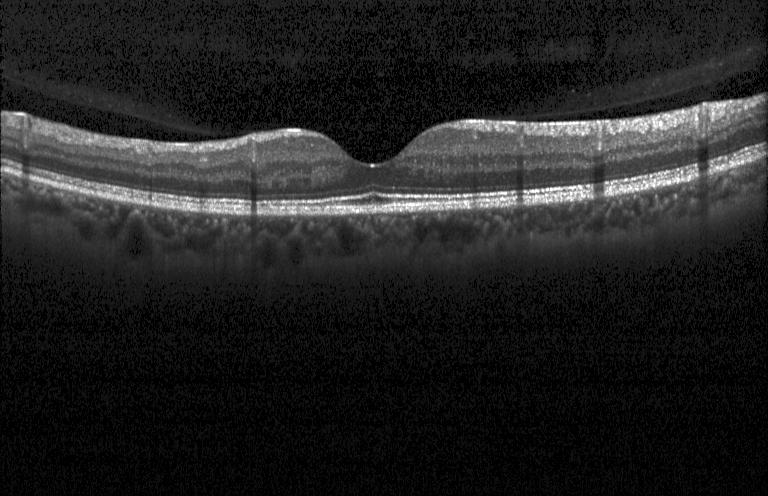 OCT B-scan showing no evidence of choroidal neovascularization, diabetic macular edema, or drusen.